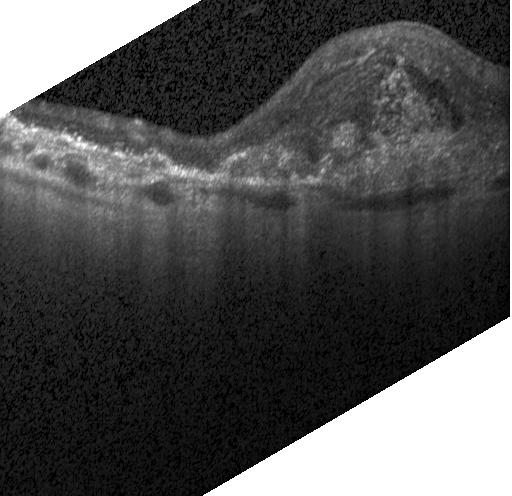

A choroidal neovascular membrane.